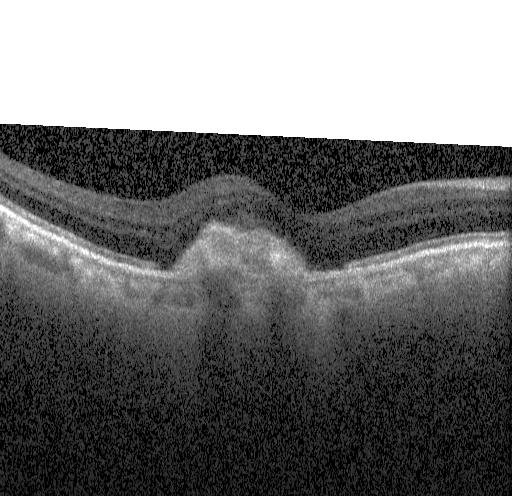
Spectral-domain OCT · optical coherence tomography scan — Finding: a choroidal neovascular membrane.